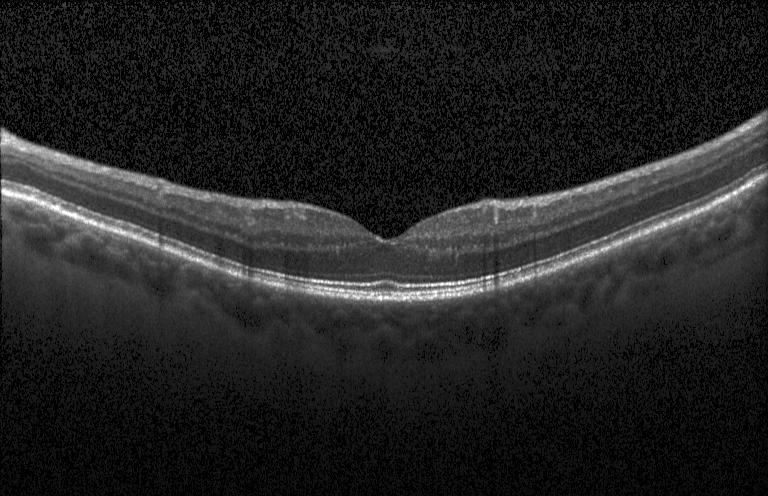 Retinal OCT cross-section, Heidelberg Spectralis OCT system
Assessment: no CNV, DME, or drusen.